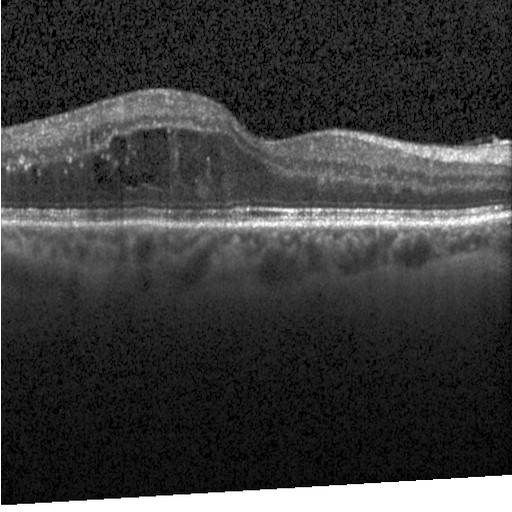
Heidelberg Spectralis, through the macula, SD-OCT, optical coherence tomography scan.
Dx: DME.